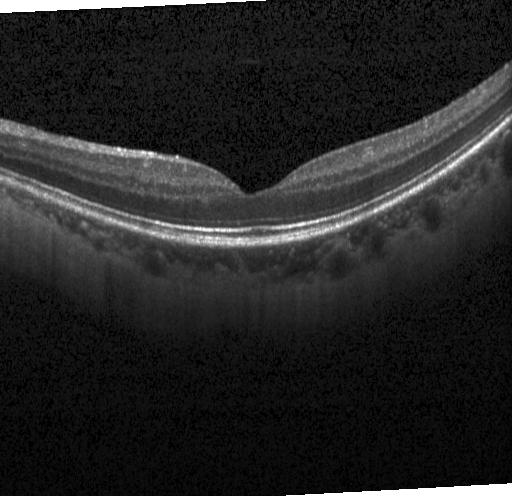
Acquired on a Heidelberg Spectralis · retinal OCT B-scan
OCT finding: neither choroidal neovascularization, diabetic macular edema, nor drusen.